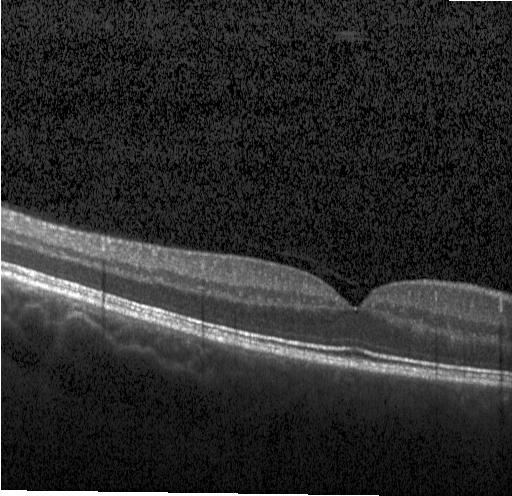 Optical coherence tomography scan. Finding: no choroidal neovascularization, no diabetic macular edema, and no drusen.